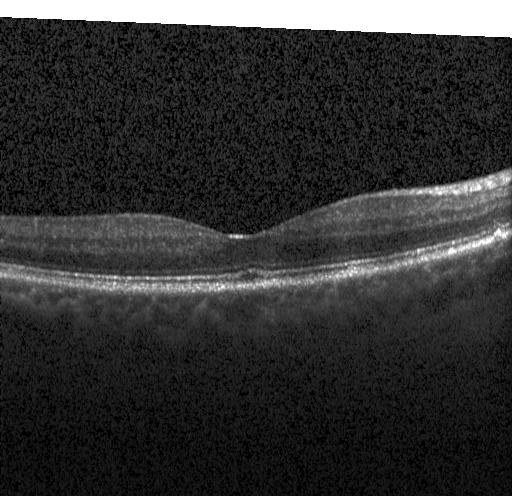

The scan shows neither CNV, DME, nor drusen.